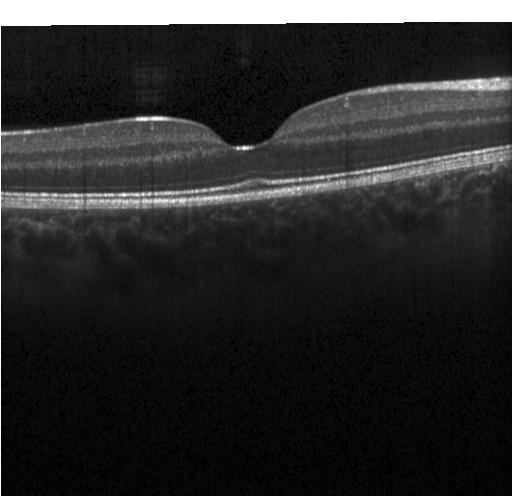
This B-scan demonstrates no choroidal neovascularization, no diabetic macular edema, and no drusen.